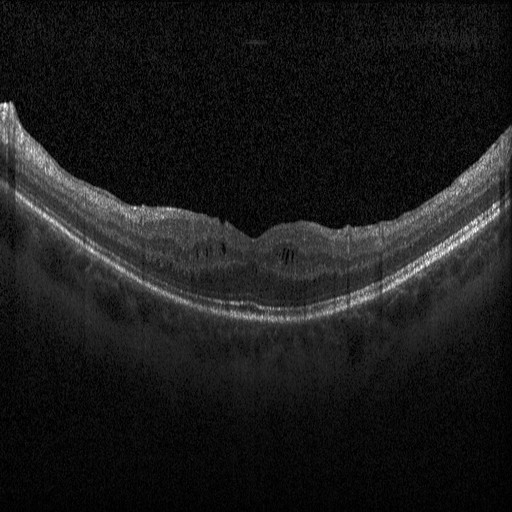

Impression: diabetic macular edema (DME).